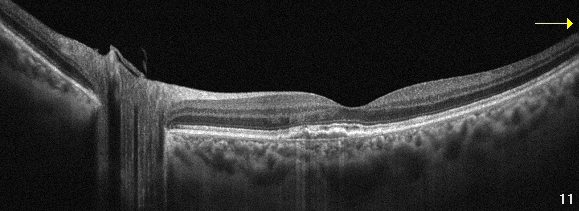
OCT line scan. Macular scan.
OCT finding: AMD.